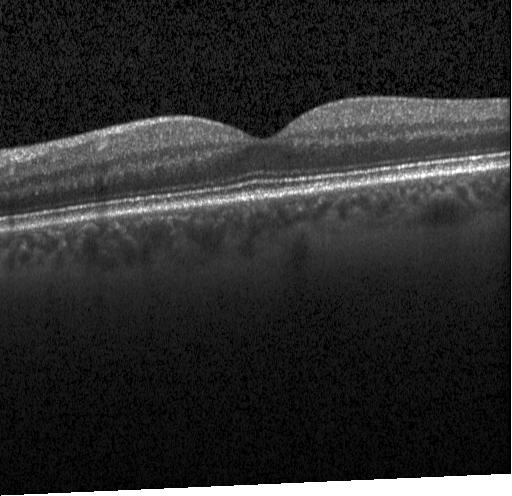 Finding: no choroidal neovascularization, no diabetic macular edema, and no drusen.